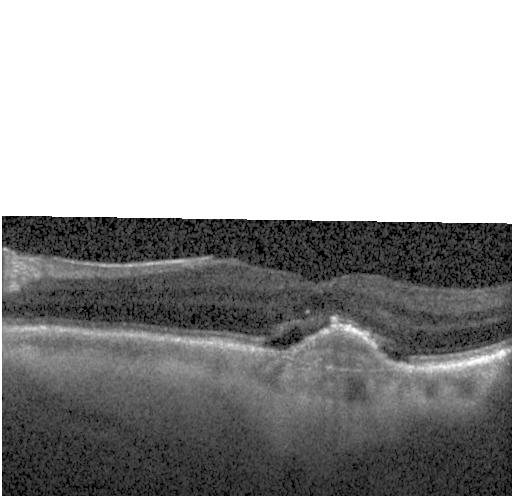
Spectral-domain optical coherence tomography. Horizontal scan through the fovea. Optical coherence tomography B-scan. Instrument: Heidelberg Spectralis
The scan shows a choroidal neovascular membrane.